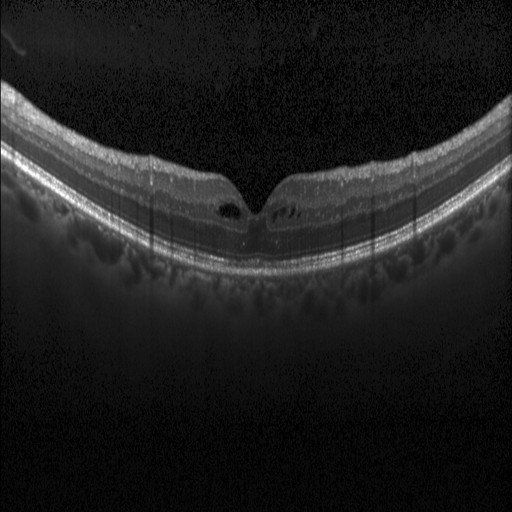
This B-scan demonstrates DME.